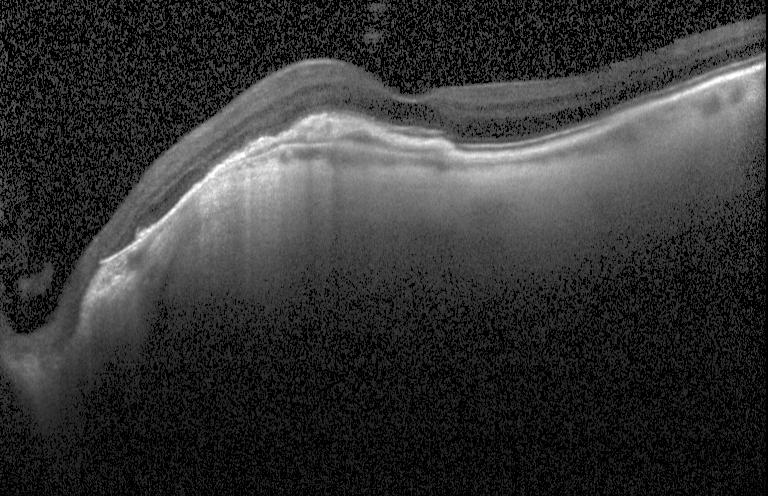
SD-OCT. Retinal OCT B-scan. Through the macula — Diagnosis: CNV.